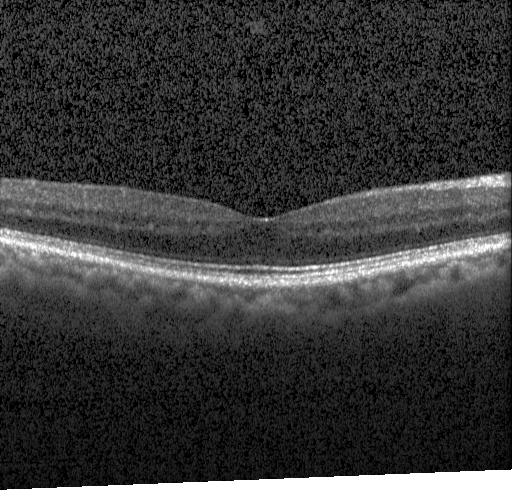
OCT line scan
Macular OCT: no CNV, DME, or drusen.